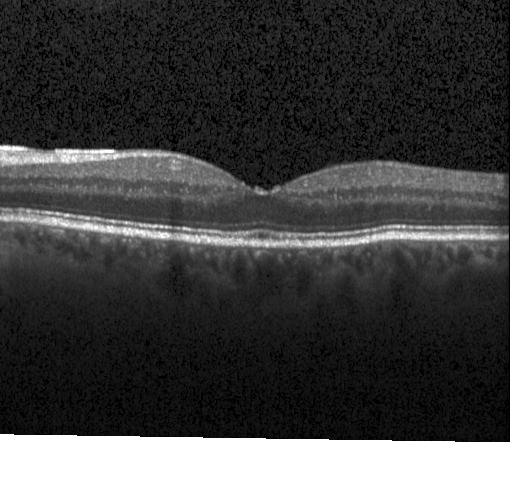

Finding: neither choroidal neovascularization, diabetic macular edema, nor drusen.